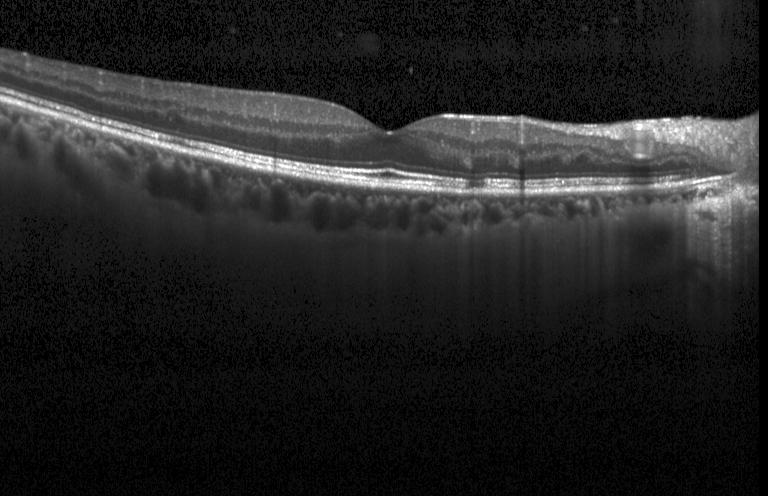

No evidence of choroidal neovascularization, diabetic macular edema, or drusen.